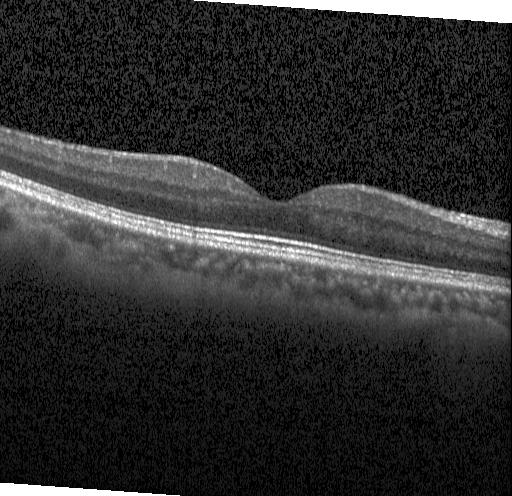
OCT finding: neither choroidal neovascularization, diabetic macular edema, nor drusen.